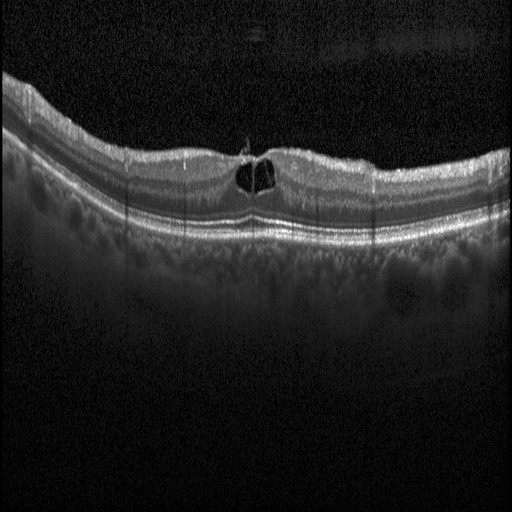

Macular OCT: diabetic macular edema (DME).